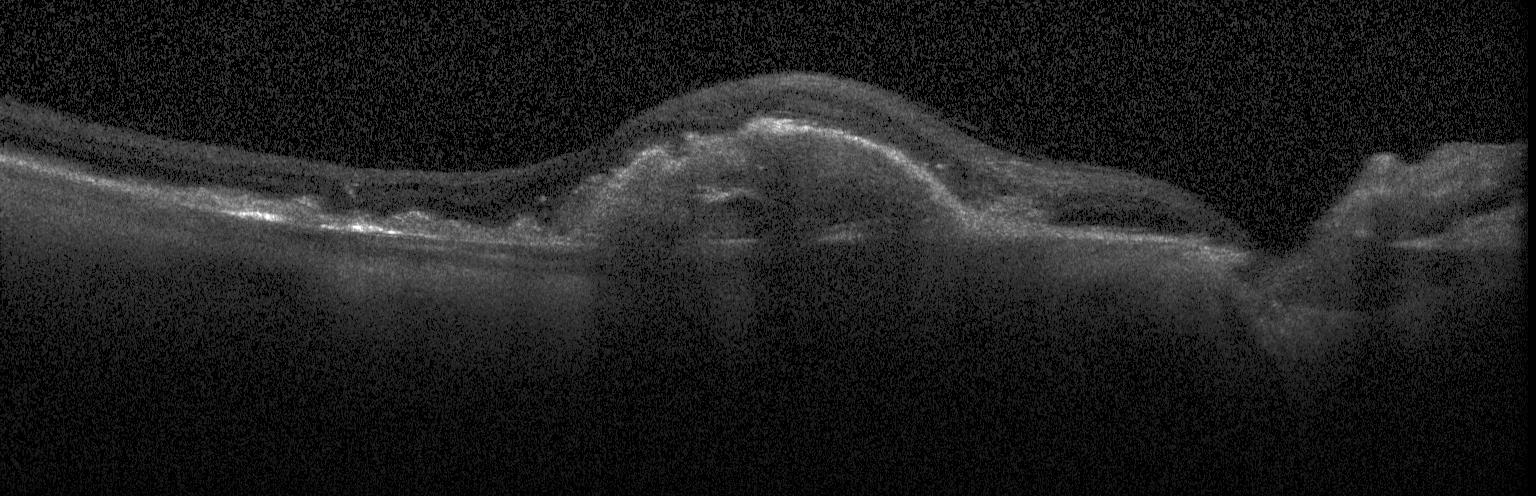
Assessment: a choroidal neovascular membrane.